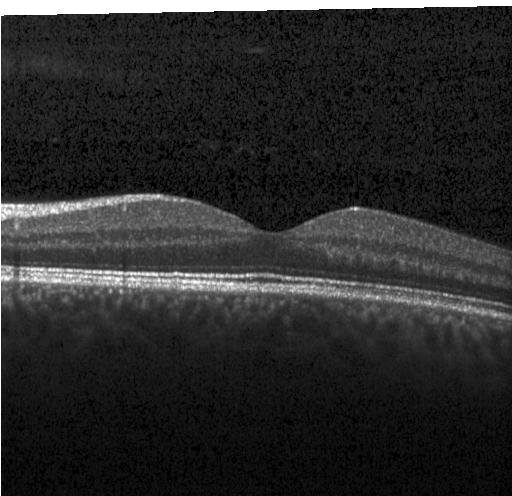

Instrument: Heidelberg Spectralis · through the macula · spectral-domain optical coherence tomography · optical coherence tomography B-scan — No CNV, no DME, and no drusen.